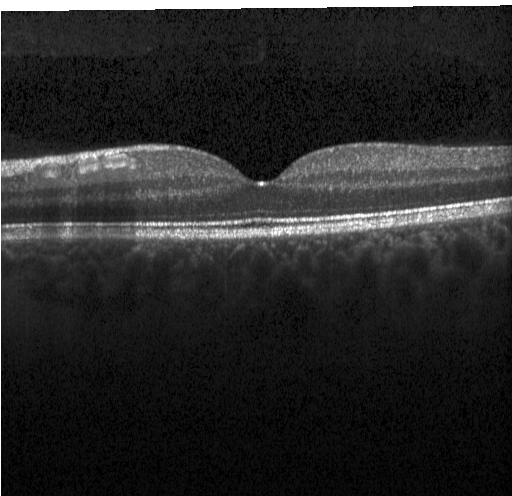
OCT finding: no evidence of choroidal neovascularization, diabetic macular edema, or drusen.